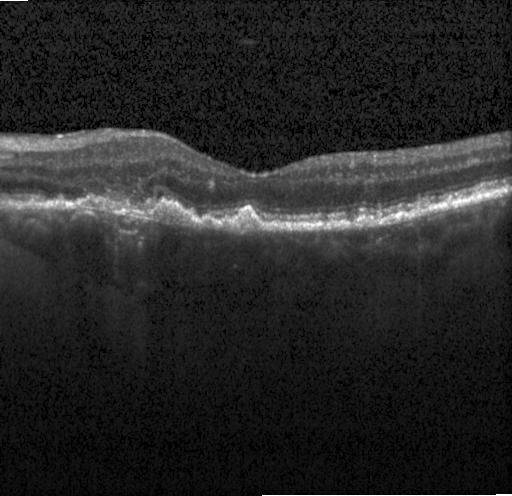 OCT line scan · spectral-domain OCT · fovea-centered. Impression: a choroidal neovascular membrane.